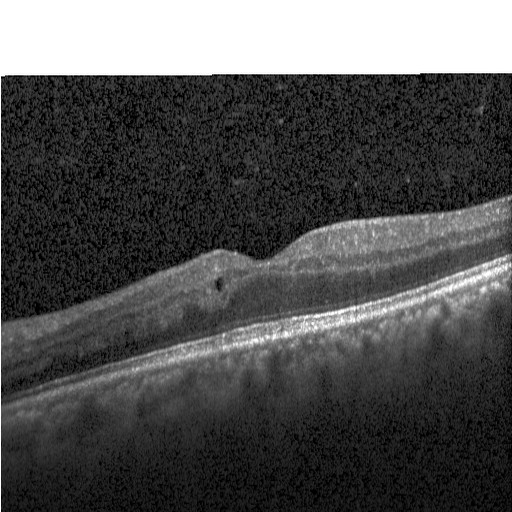
Spectral-domain optical coherence tomography, optical coherence tomography B-scan. Macular OCT: diabetic macular edema.